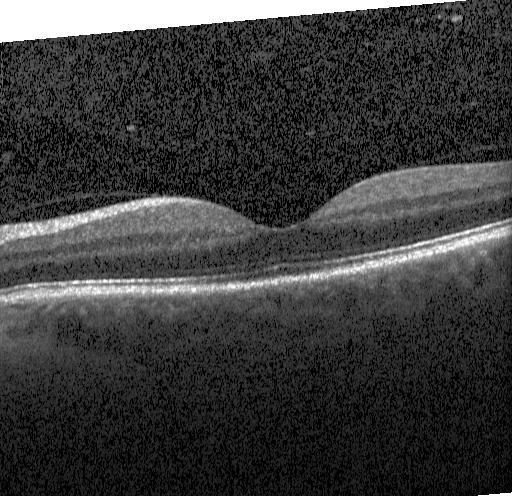 Macular OCT demonstrating neither CNV, DME, nor drusen.